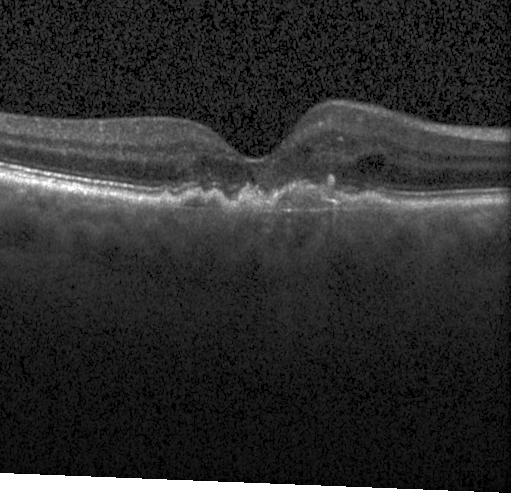
Retinal OCT B-scan — Finding: choroidal neovascularization.